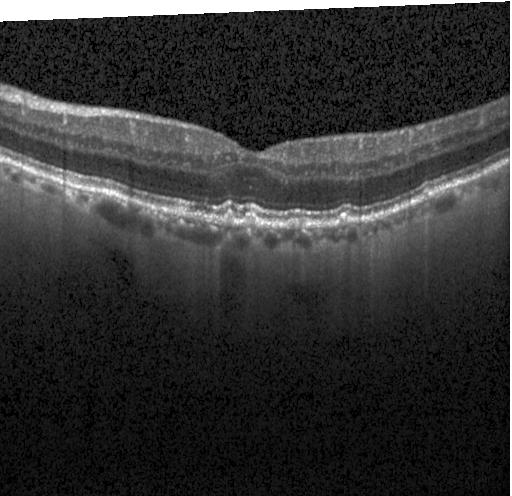
Optical coherence tomography B-scan. This B-scan demonstrates sub-RPE drusenoid deposits.